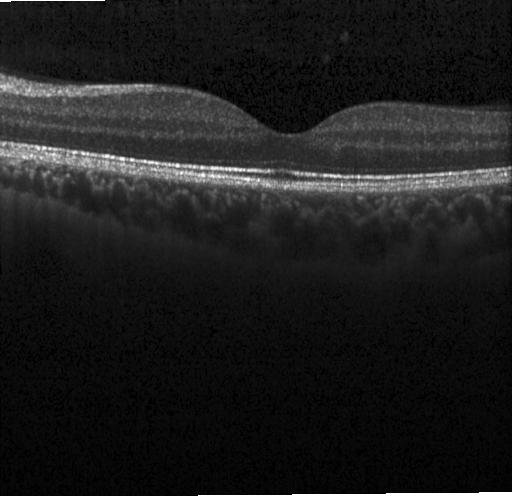 Spectral-domain OCT B-scan: no choroidal neovascularization, no diabetic macular edema, and no drusen.